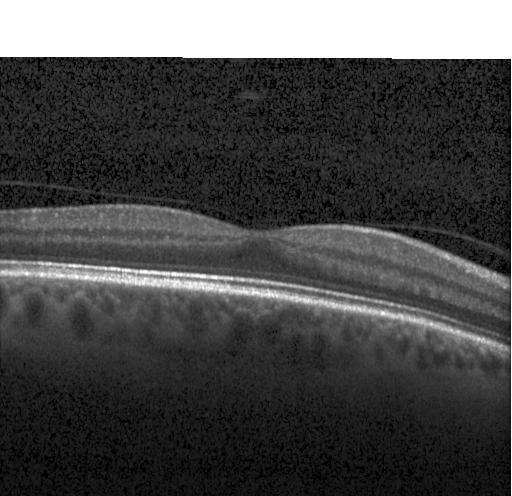
This B-scan demonstrates no evidence of CNV, DME, or drusen.